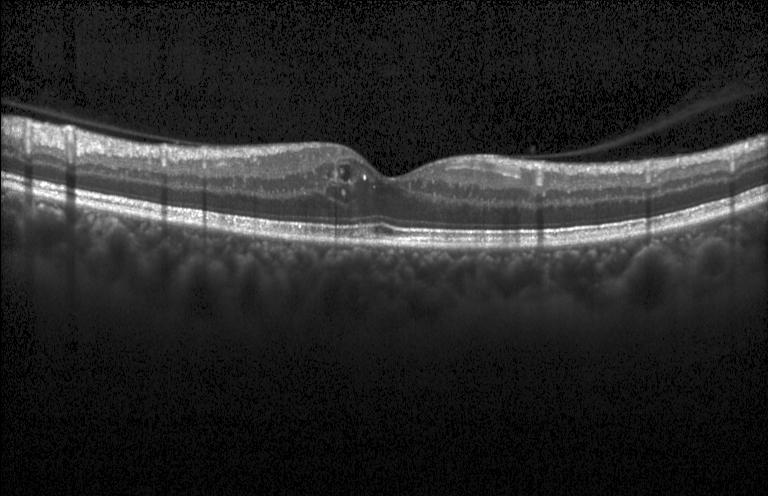 OCT line scan. Acquired on a Heidelberg Spectralis. Spectral-domain optical coherence tomography
Assessment: diabetic macular edema (DME).